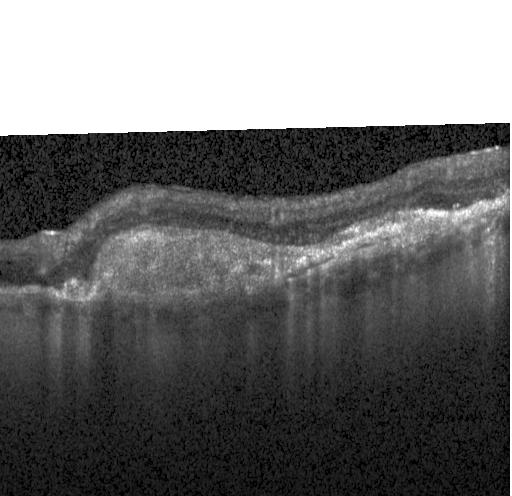

Finding: a choroidal neovascular membrane.